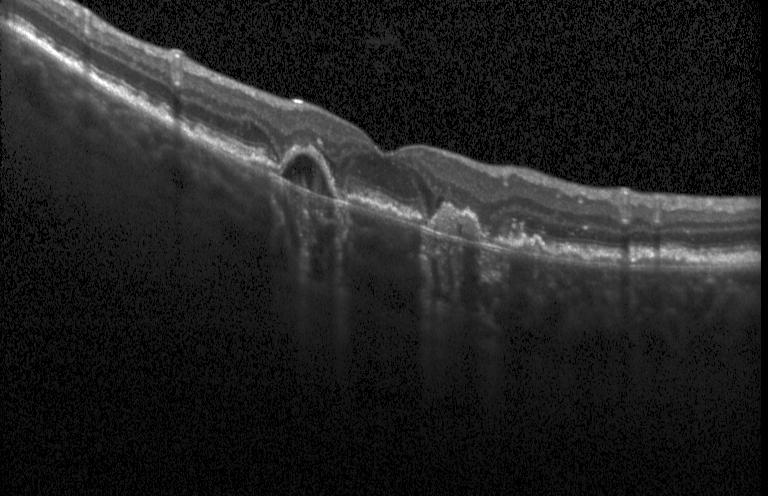

Finding: a choroidal neovascular membrane.